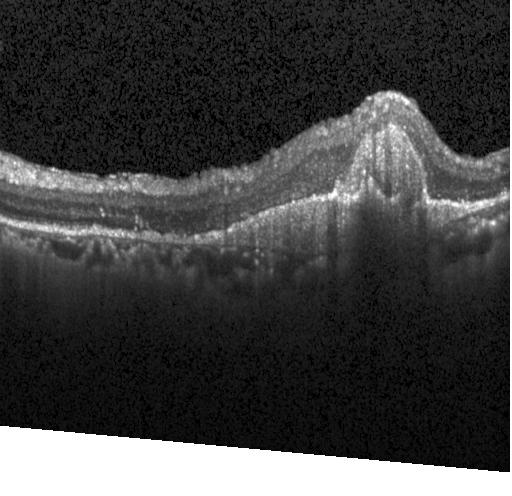 Horizontal scan through the fovea; acquired on a Heidelberg Spectralis; spectral-domain OCT; OCT line scan. The scan shows choroidal neovascularization.